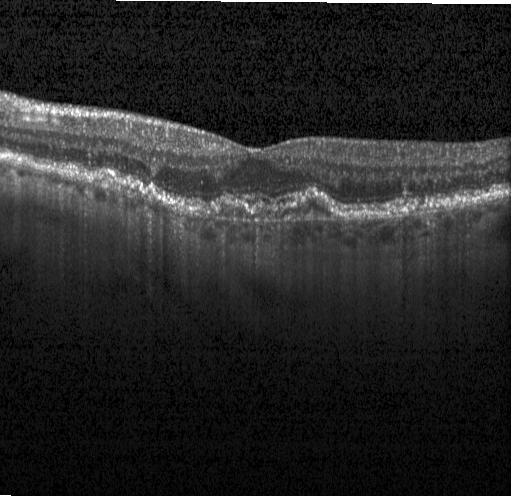

Retinal OCT cross-section; instrument: Heidelberg Spectralis
Impression: a choroidal neovascular membrane.